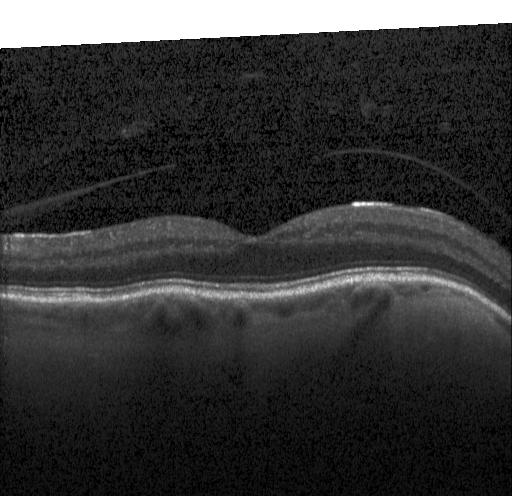

Heidelberg Spectralis OCT system, SD-OCT, macular scan, optical coherence tomography B-scan. Diagnosis: neither choroidal neovascularization, diabetic macular edema, nor drusen.